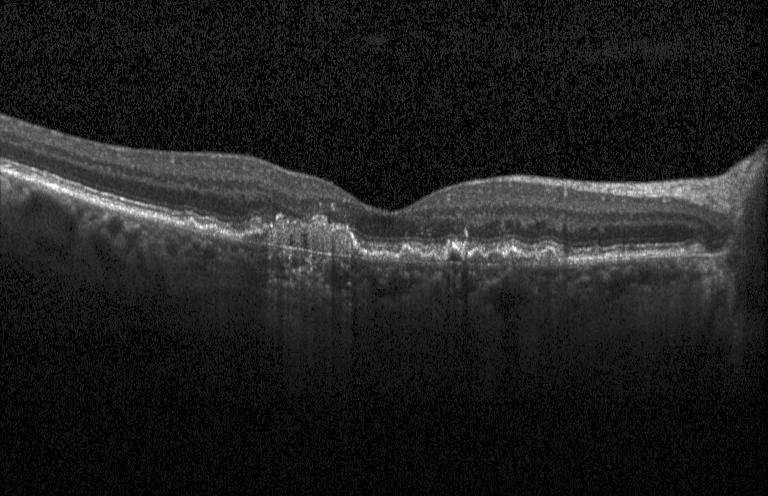 Diagnosis: a choroidal neovascular membrane.